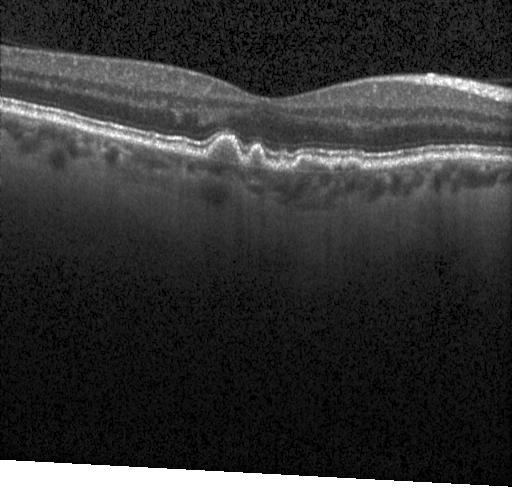 OCT B-scan showing sub-RPE drusenoid deposits.